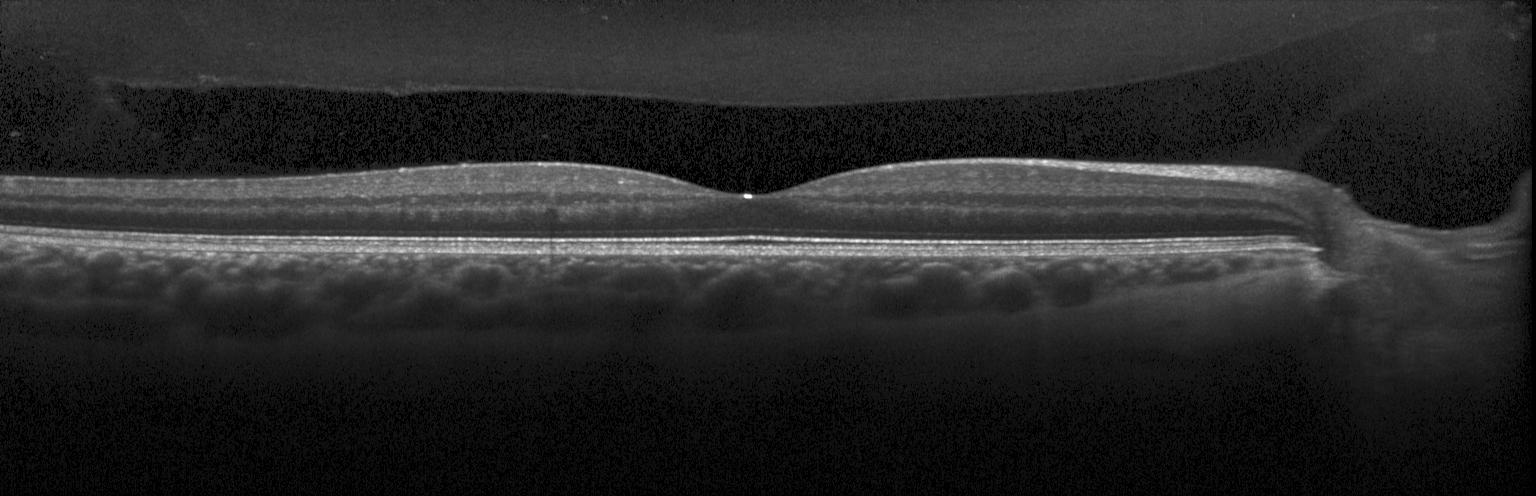 Finding: neither choroidal neovascularization, diabetic macular edema, nor drusen.